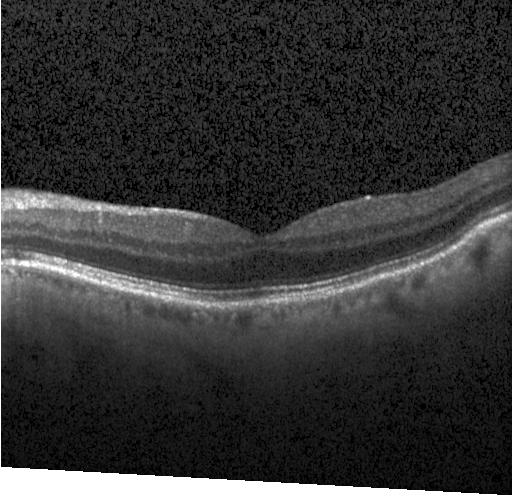 Spectral-domain optical coherence tomography. Macular scan. Retinal OCT B-scan. Instrument: Heidelberg Spectralis.
No CNV, no DME, and no drusen.